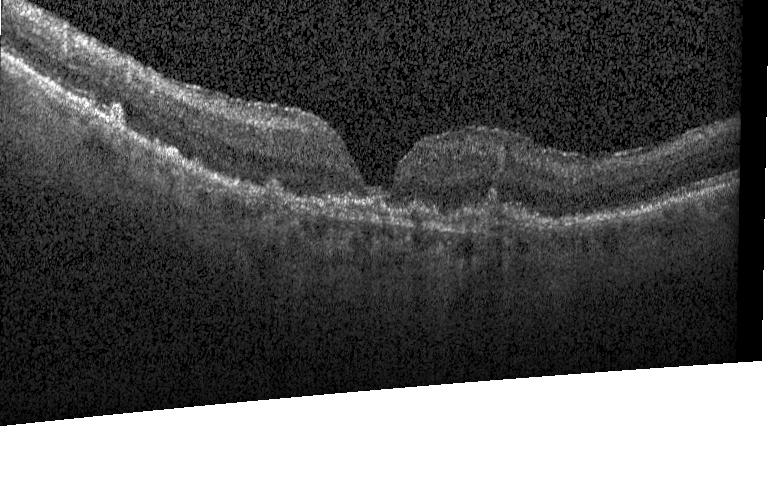 Acquired on a Heidelberg Spectralis. Through the macula. OCT B-scan. SD-OCT — This B-scan demonstrates choroidal neovascularization (CNV).